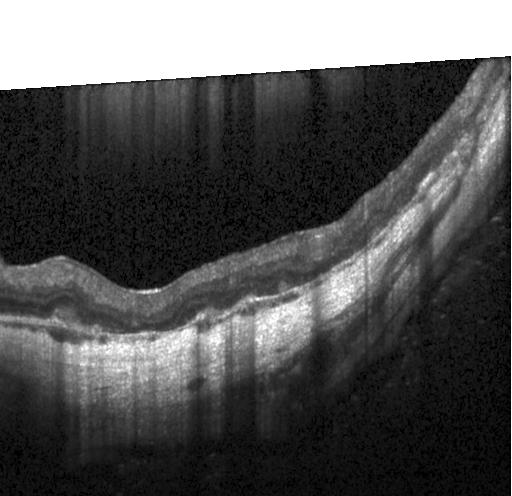 Dx: CNV.